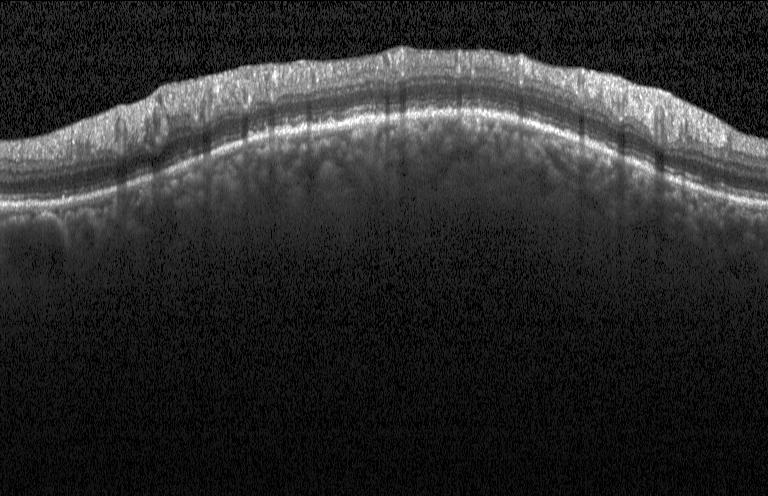

OCT line scan, instrument: Heidelberg Spectralis. Finding: a choroidal neovascular membrane.